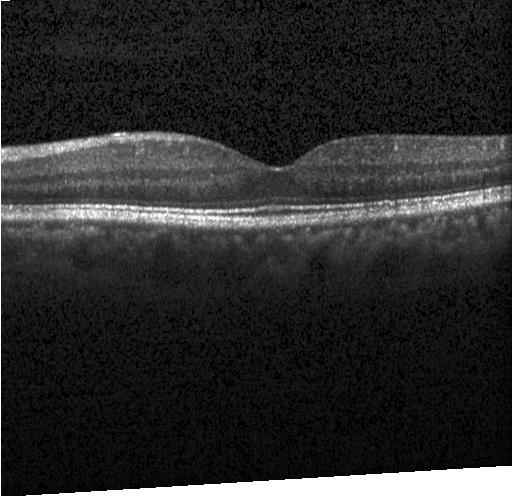

OCT B-scan, fovea-centered
OCT finding: neither choroidal neovascularization, diabetic macular edema, nor drusen.